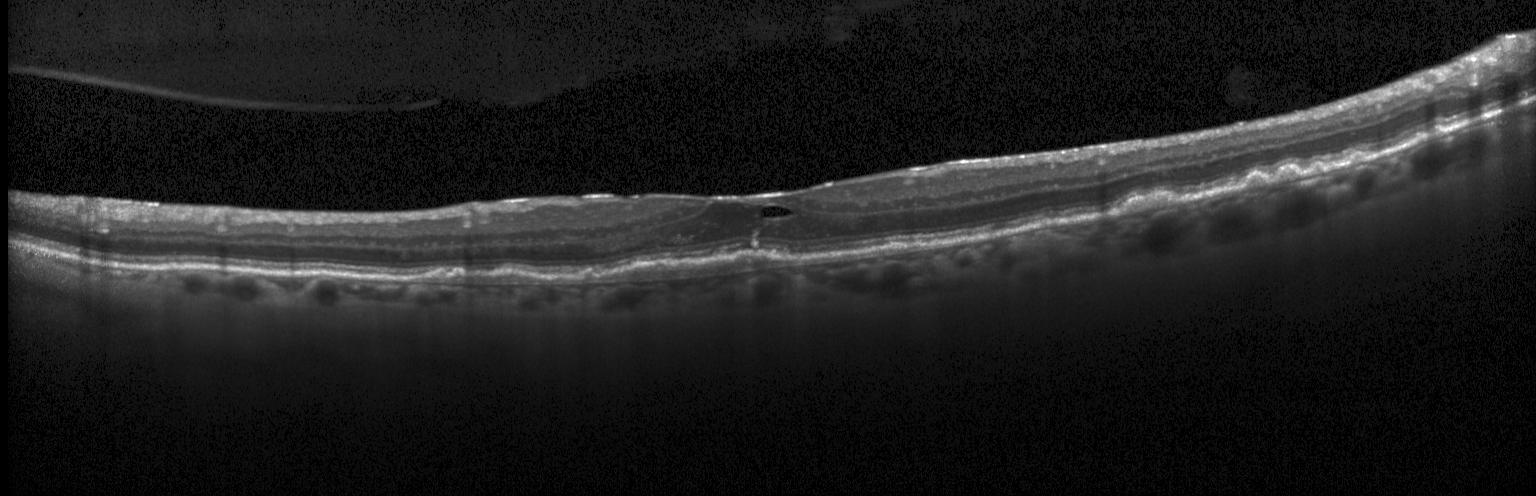
Optical coherence tomography scan. Finding: a choroidal neovascular membrane.